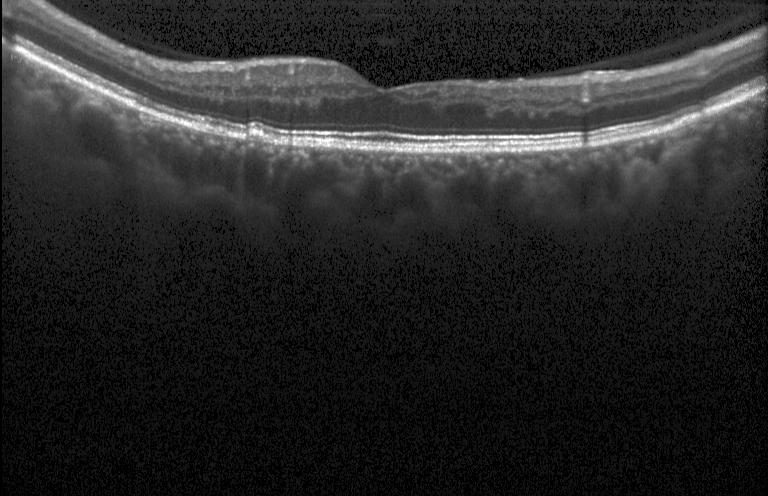

Retinal OCT cross-section. Instrument: Heidelberg Spectralis. Spectral-domain OCT. Dx: multiple drusen.